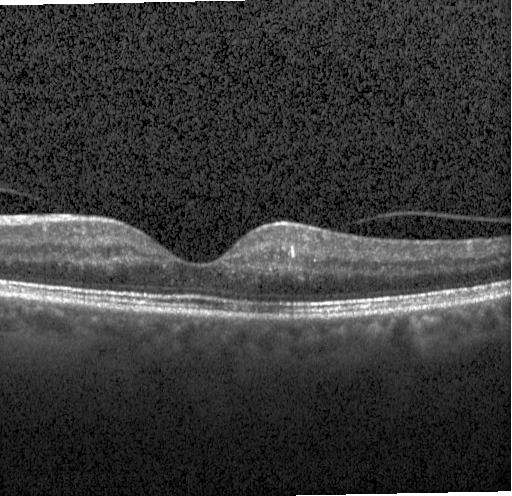
Optical coherence tomography B-scan
Finding: no evidence of choroidal neovascularization, diabetic macular edema, or drusen.